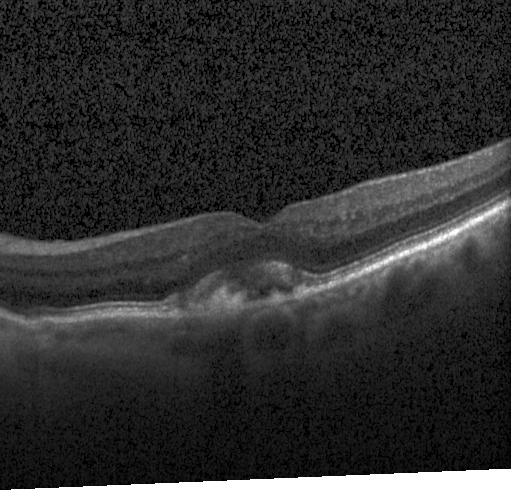

Centered on the fovea · acquired on a Heidelberg Spectralis · spectral-domain optical coherence tomography · retinal OCT cross-section
Diagnosis: a choroidal neovascular membrane.